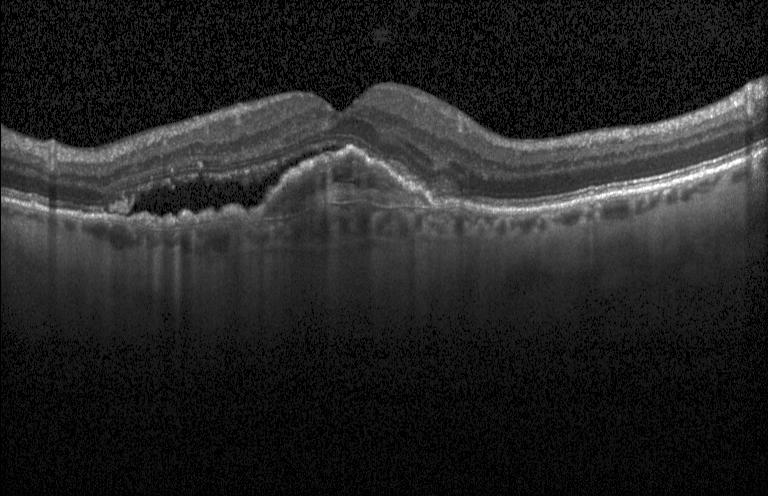
Impression: a choroidal neovascular membrane.